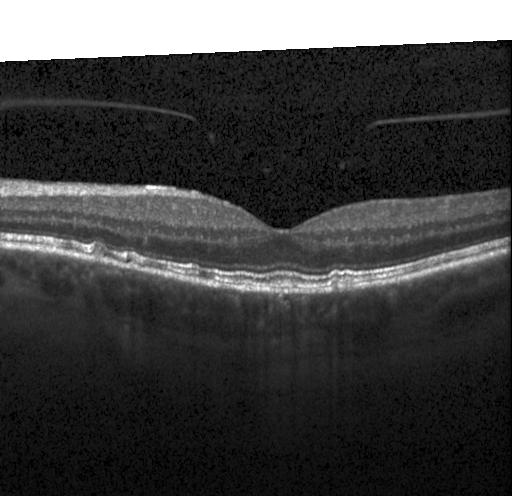

Instrument: Heidelberg Spectralis, SD-OCT, macular scan, optical coherence tomography scan
OCT finding: multiple drusen.